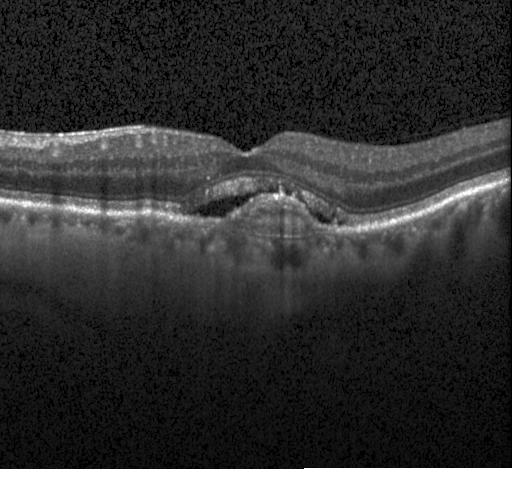
OCT B-scan — OCT finding: choroidal neovascularization.